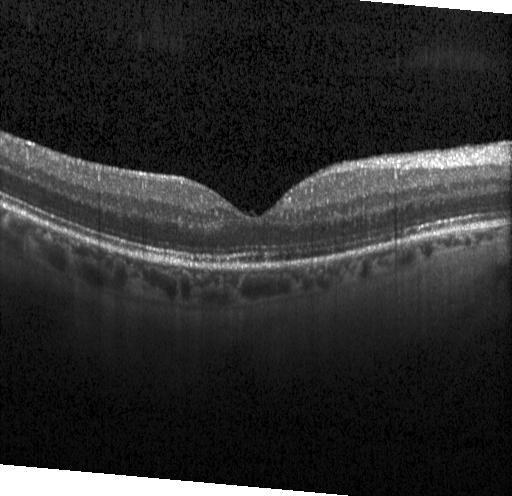

OCT B-scan, instrument: Heidelberg Spectralis.
The scan shows neither choroidal neovascularization, diabetic macular edema, nor drusen.